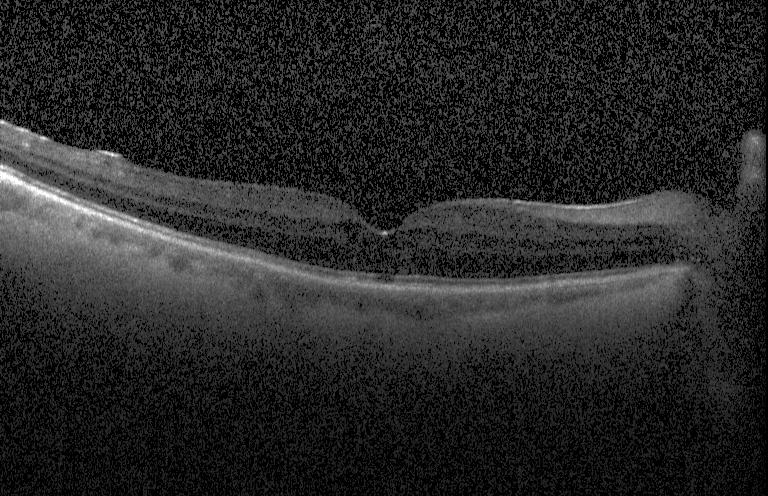
Heidelberg Spectralis, retinal OCT cross-section. No evidence of choroidal neovascularization, diabetic macular edema, or drusen.